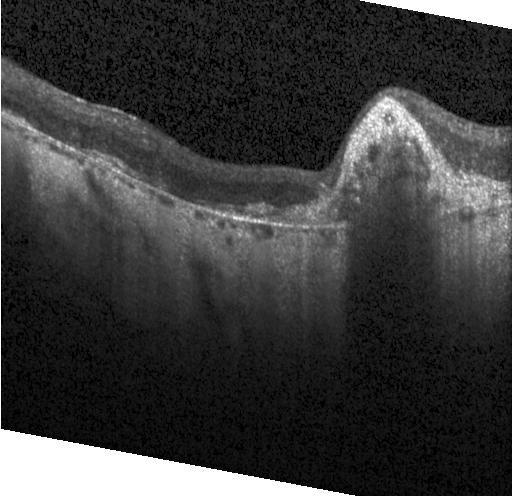 Instrument: Heidelberg Spectralis, macular scan, OCT B-scan.
Diagnosis: CNV.